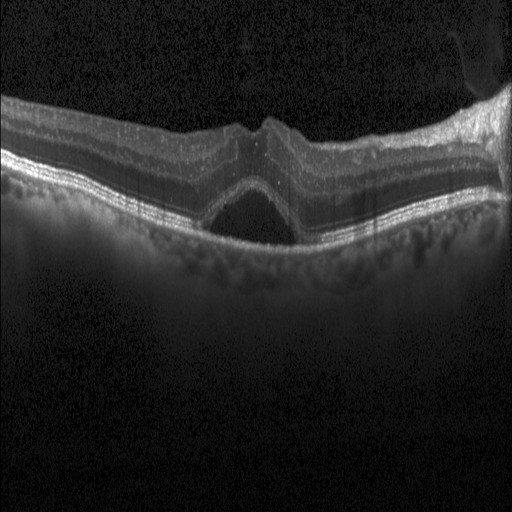
Spectral-domain OCT. Retinal OCT B-scan. Instrument: Heidelberg Spectralis. Horizontal scan through the fovea
Diagnosis: DME.